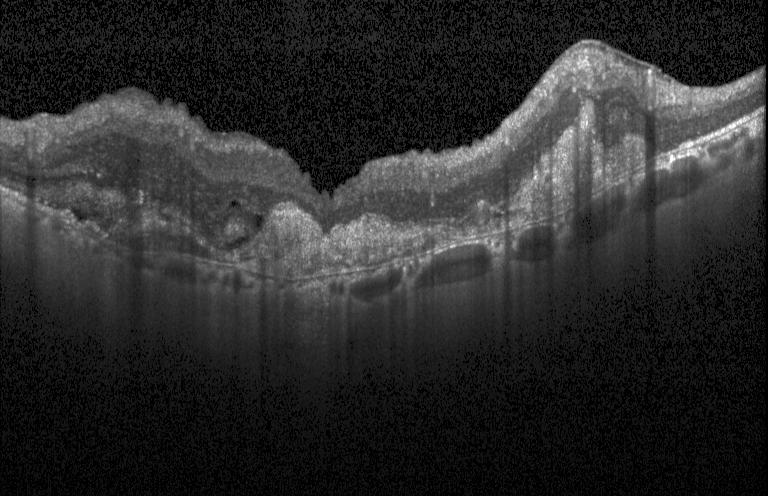

Retinal OCT B-scan · SD-OCT · macular scan. The scan shows choroidal neovascularization.